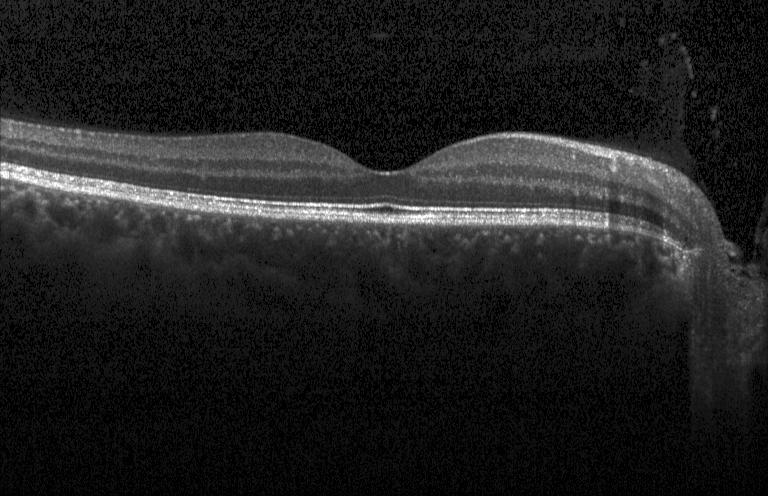
Instrument: Heidelberg Spectralis, retinal OCT cross-section, SD-OCT, through the macula — OCT finding: no evidence of choroidal neovascularization, diabetic macular edema, or drusen.